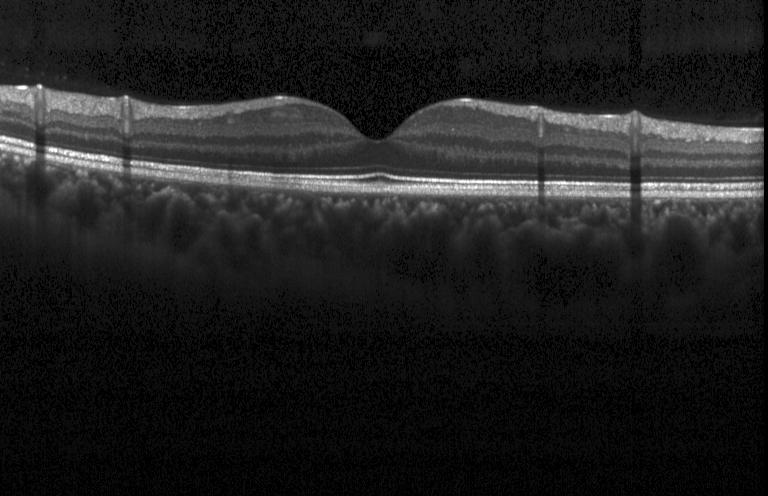 Acquired on a Heidelberg Spectralis; OCT B-scan.
Impression: neither CNV, DME, nor drusen.